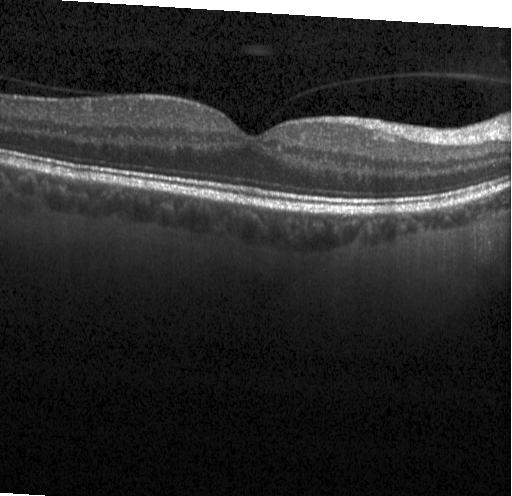
Macular OCT: no CNV, no DME, and no drusen.